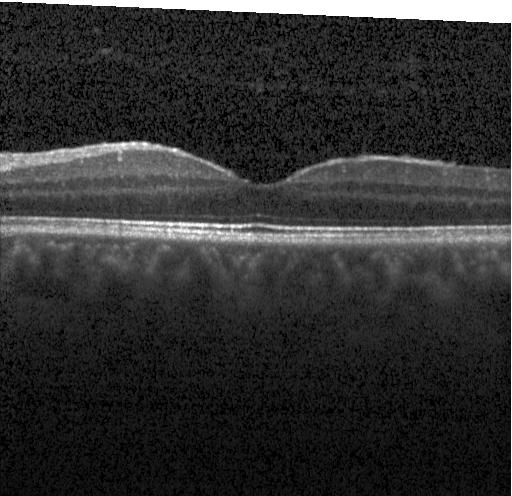 Dx: no choroidal neovascularization, no diabetic macular edema, and no drusen.